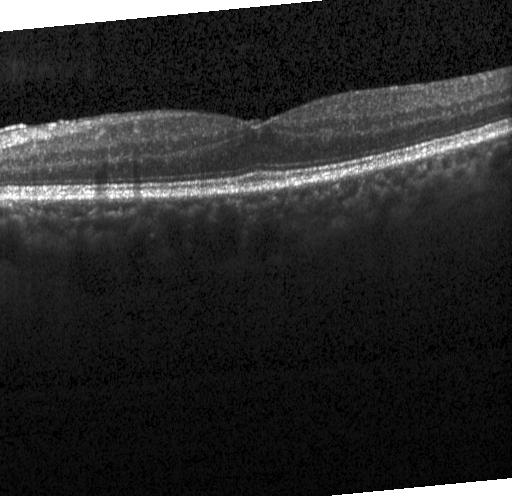 Spectral-domain OCT; retinal OCT cross-section. This B-scan demonstrates no choroidal neovascularization, no diabetic macular edema, and no drusen.